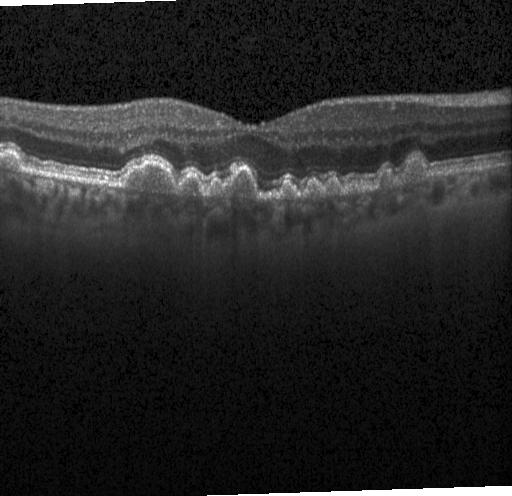 OCT B-scan
Dx: drusen.